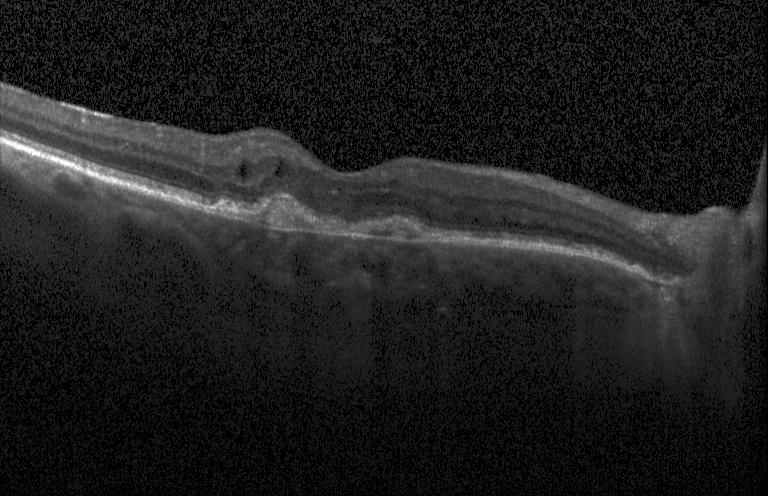 Diagnosis: a choroidal neovascular membrane.